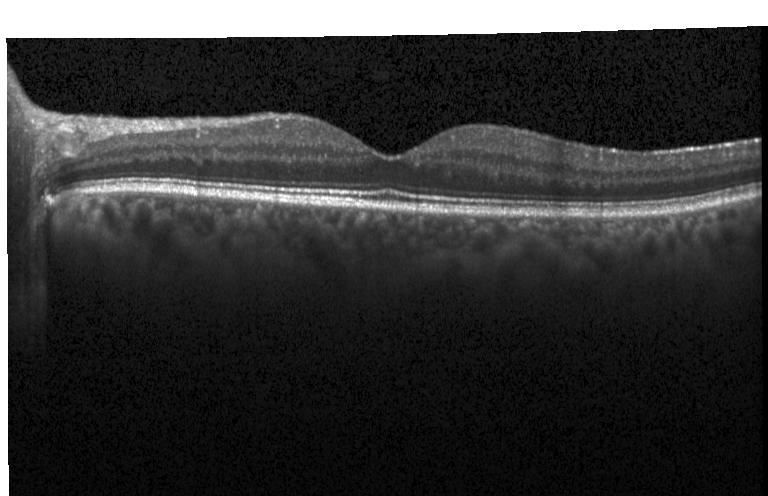

OCT B-scan. Spectral-domain optical coherence tomography
OCT finding: no choroidal neovascularization, diabetic macular edema, or drusen.